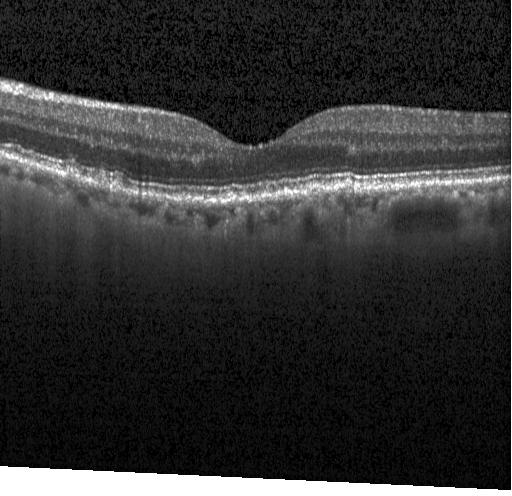

Horizontal scan through the fovea · SD-OCT · optical coherence tomography B-scan. Finding: multiple drusen.